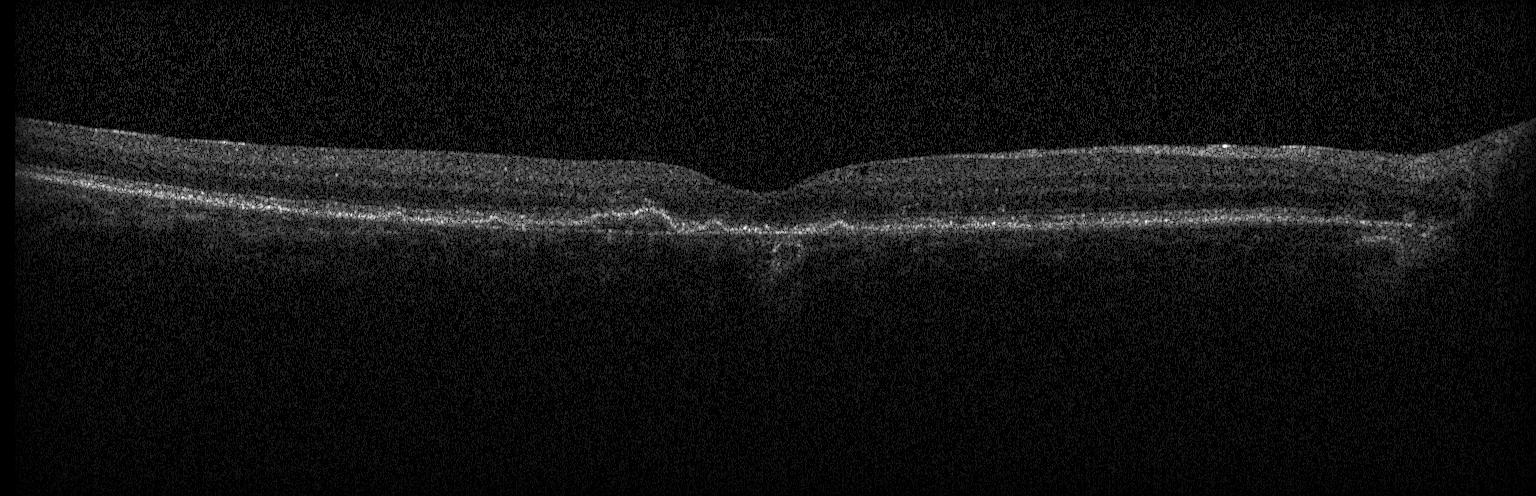
Retinal OCT cross-section showing a choroidal neovascular membrane.